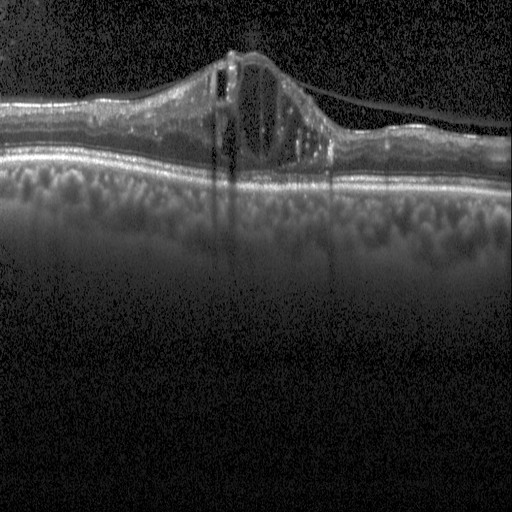

Spectral-domain OCT B-scan: DME.